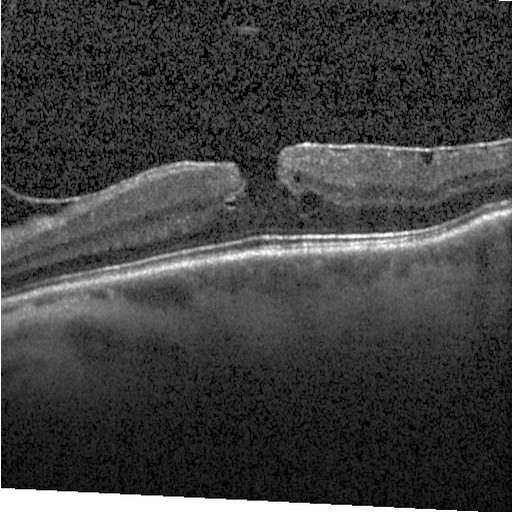

This B-scan demonstrates diabetic macular edema.